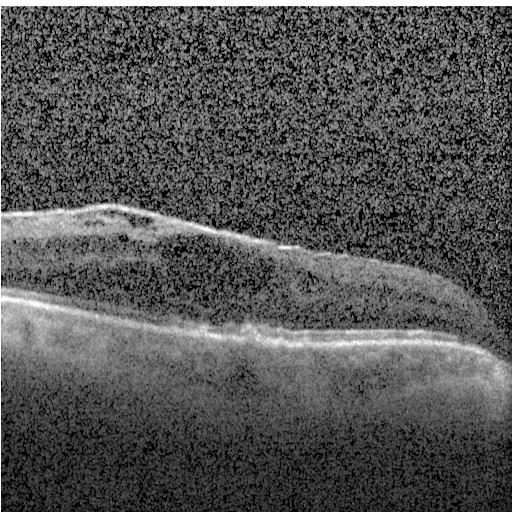

Diagnosis: diabetic macular edema.